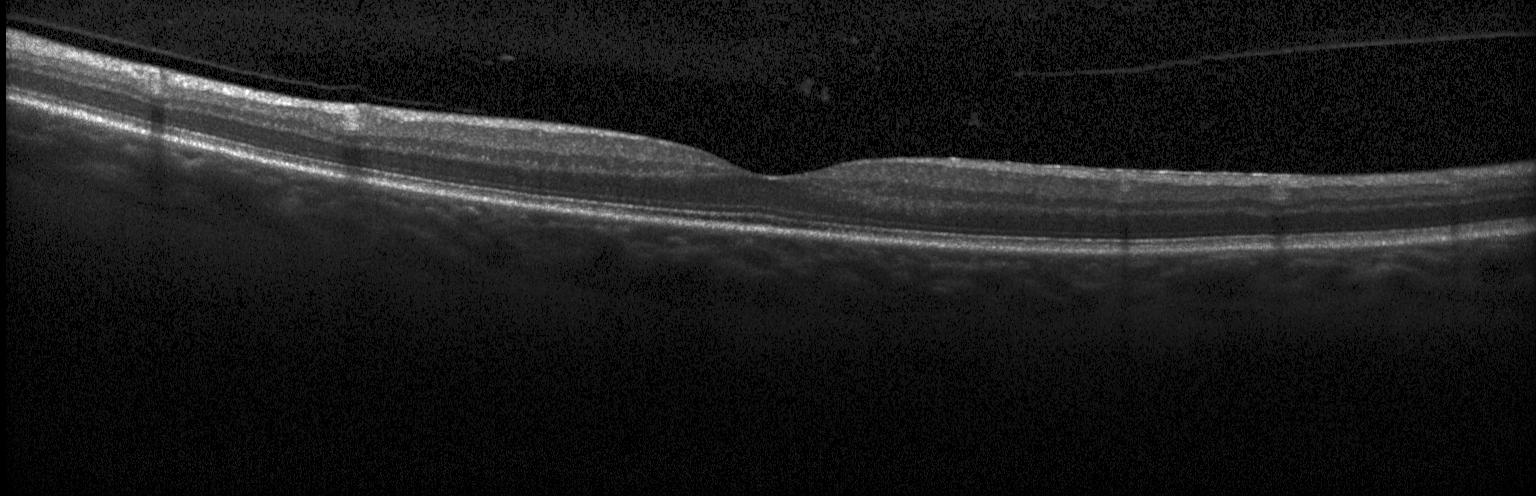 Optical coherence tomography B-scan; SD-OCT; fovea-centered; Heidelberg Spectralis. This B-scan demonstrates no choroidal neovascularization, no diabetic macular edema, and no drusen.